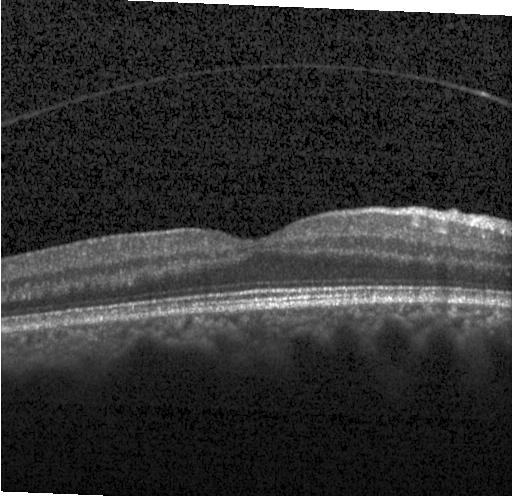 Centered on the fovea · acquired on a Heidelberg Spectralis · retinal OCT cross-section.
Assessment: no choroidal neovascularization, no diabetic macular edema, and no drusen.